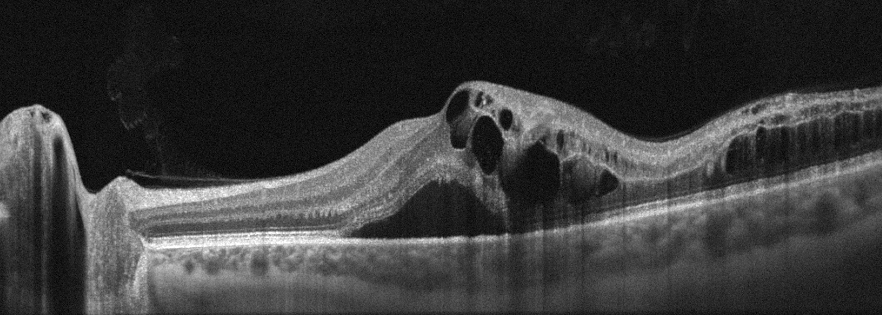

Finding: retinal vein occlusion (RVO).